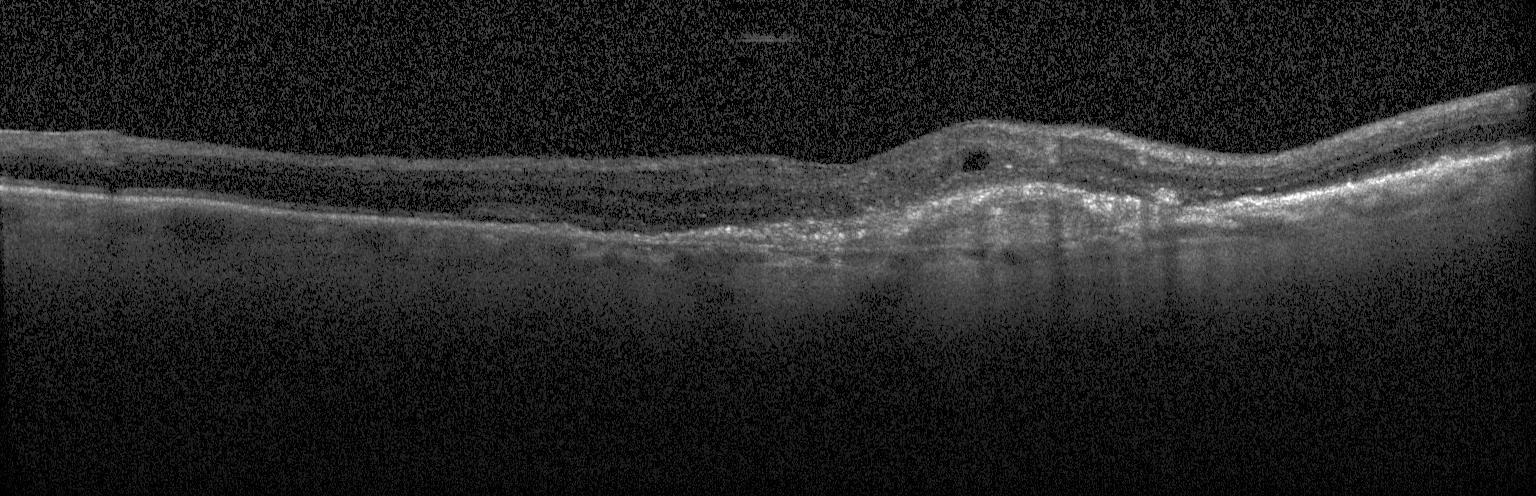

OCT line scan; horizontal scan through the fovea; acquired on a Heidelberg Spectralis; SD-OCT
A choroidal neovascular membrane.